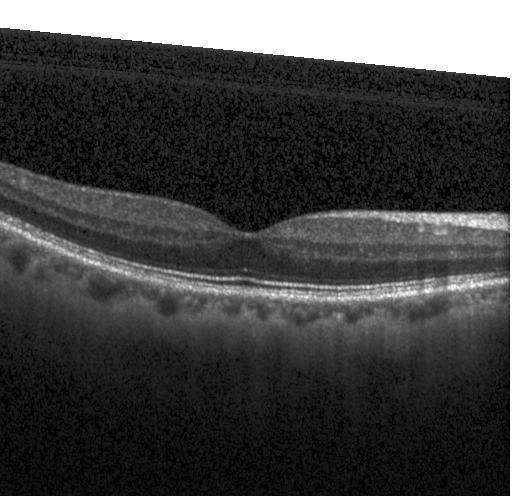

OCT line scan.
No evidence of choroidal neovascularization, diabetic macular edema, or drusen.